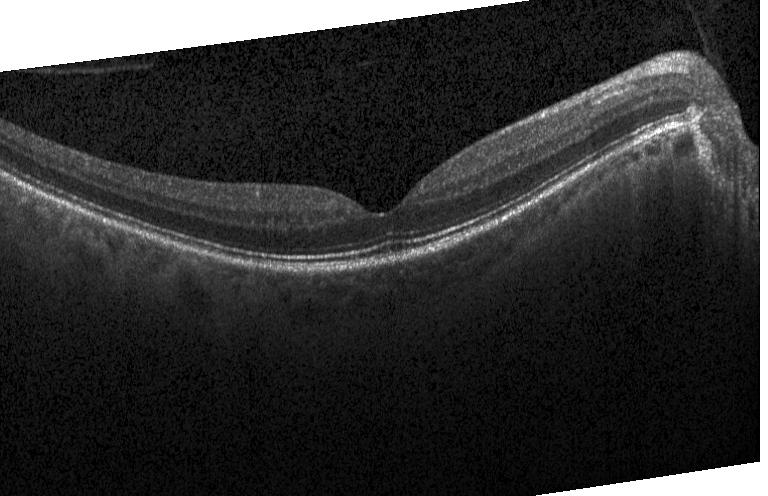

Optical coherence tomography scan. Horizontal scan through the fovea. Heidelberg Spectralis OCT system. SD-OCT. Finding: no evidence of choroidal neovascularization, diabetic macular edema, or drusen.